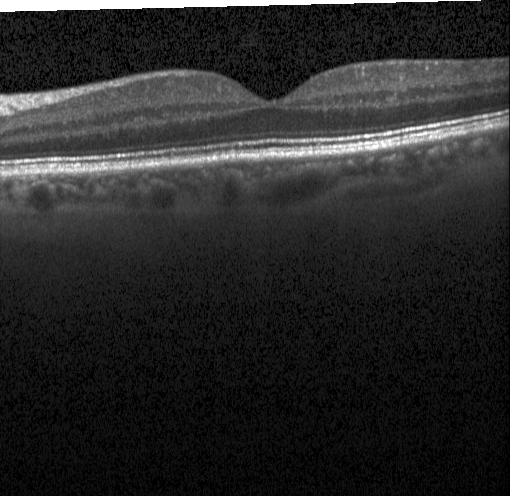

Diagnosis: neither choroidal neovascularization, diabetic macular edema, nor drusen.